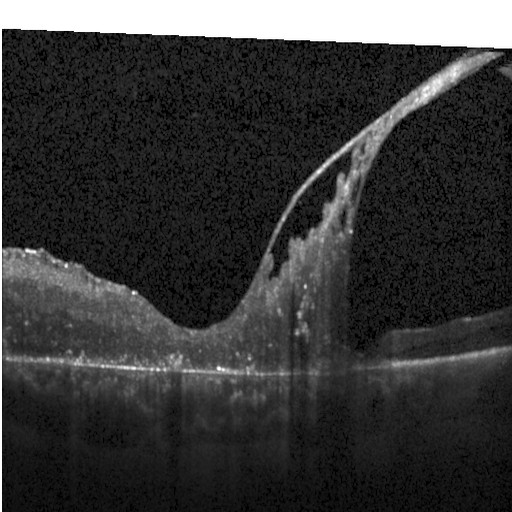 Spectral-domain OCT B-scan: diabetic macular edema (DME).